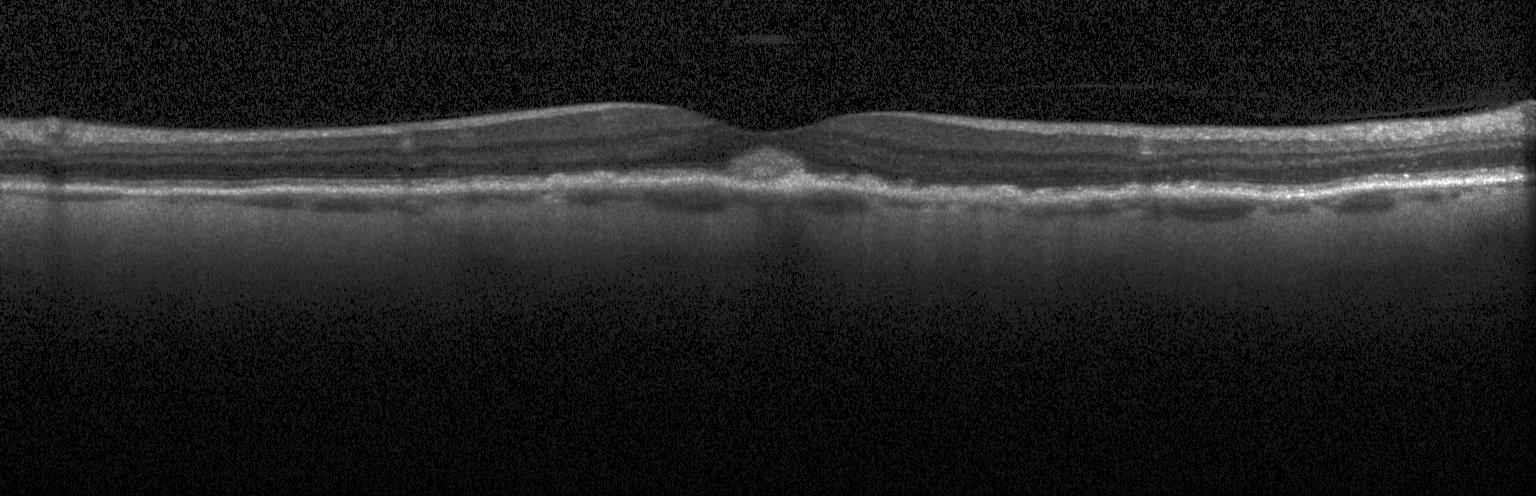 Instrument: Heidelberg Spectralis, retinal OCT B-scan, spectral-domain optical coherence tomography — Finding: sub-RPE drusenoid deposits.